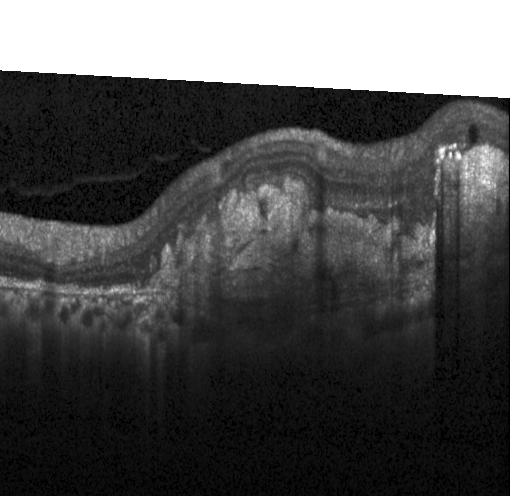

Dx: a choroidal neovascular membrane.